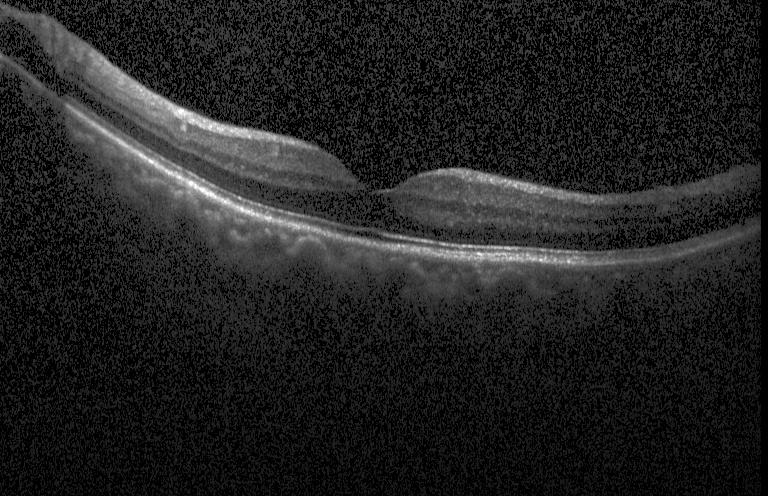 Spectral-domain OCT B-scan: no CNV, no DME, and no drusen.